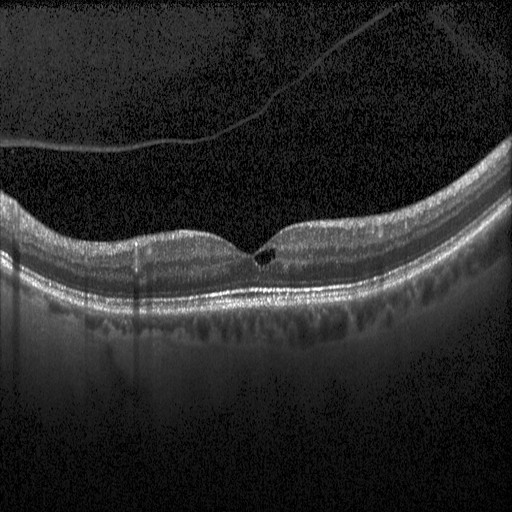
OCT B-scan · centered on the fovea — This B-scan demonstrates diabetic macular edema (DME).